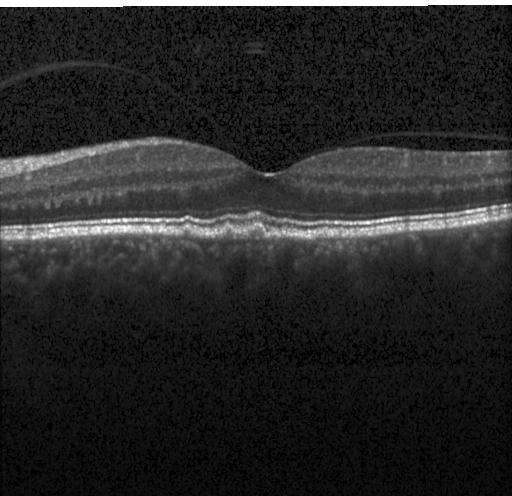 OCT B-scan · macular scan · Heidelberg Spectralis
Impression: drusen.